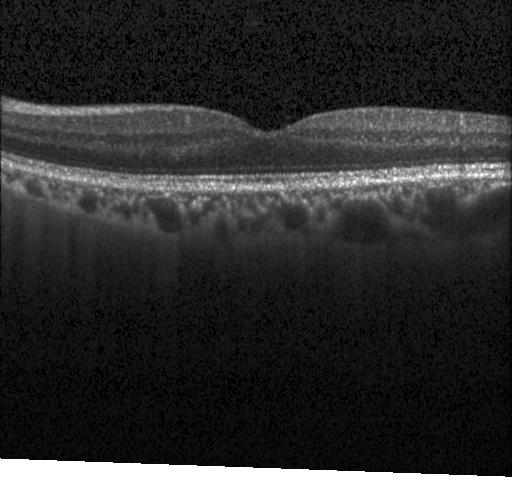 Horizontal scan through the fovea, instrument: Heidelberg Spectralis, spectral-domain OCT, OCT B-scan.
Impression: no choroidal neovascularization, no diabetic macular edema, and no drusen.